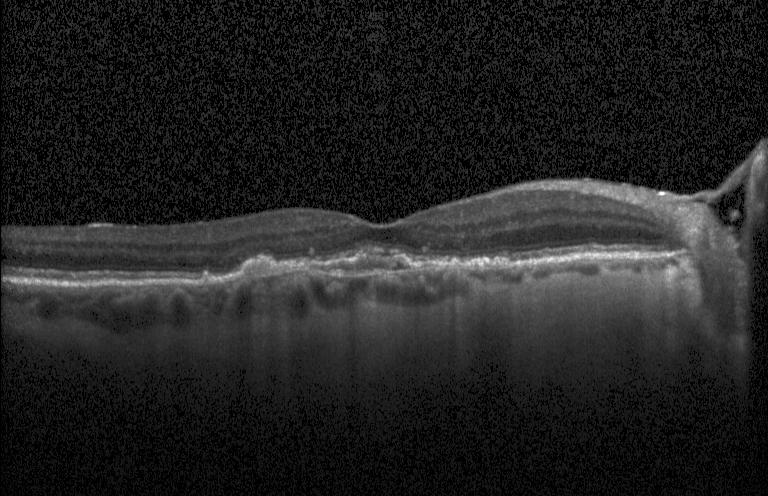 SD-OCT; centered on the fovea; Heidelberg Spectralis OCT system; retinal OCT cross-section. Macular OCT: choroidal neovascularization.